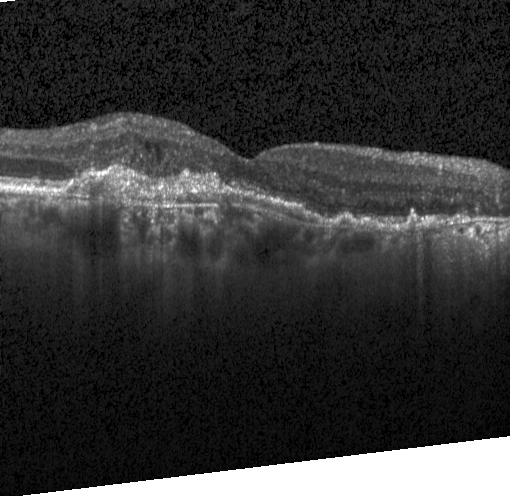
Spectral-domain OCT; Heidelberg Spectralis; retinal OCT B-scan.
Finding: a choroidal neovascular membrane.